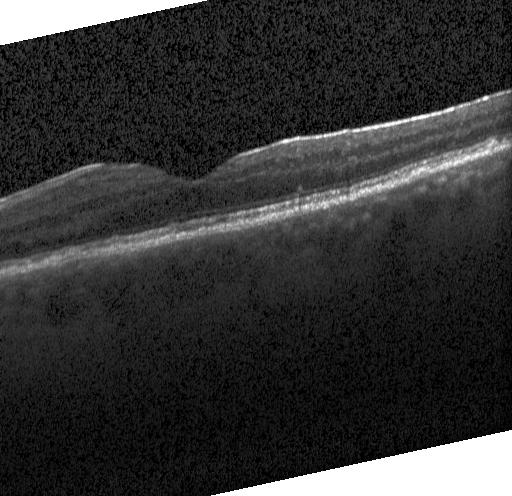
Horizontal scan through the fovea · instrument: Heidelberg Spectralis · spectral-domain optical coherence tomography · retinal OCT cross-section — Dx: no evidence of choroidal neovascularization, diabetic macular edema, or drusen.